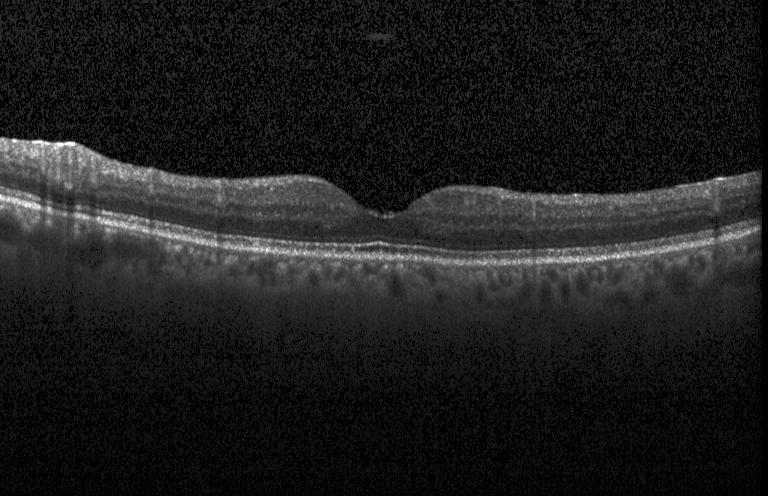 Instrument: Heidelberg Spectralis; macular scan; spectral-domain optical coherence tomography; OCT line scan — The scan shows no choroidal neovascularization, no diabetic macular edema, and no drusen.